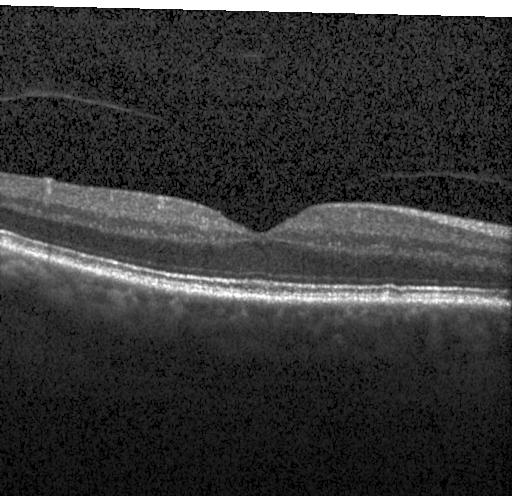

SD-OCT, optical coherence tomography B-scan, Heidelberg Spectralis OCT system
Neither choroidal neovascularization, diabetic macular edema, nor drusen.